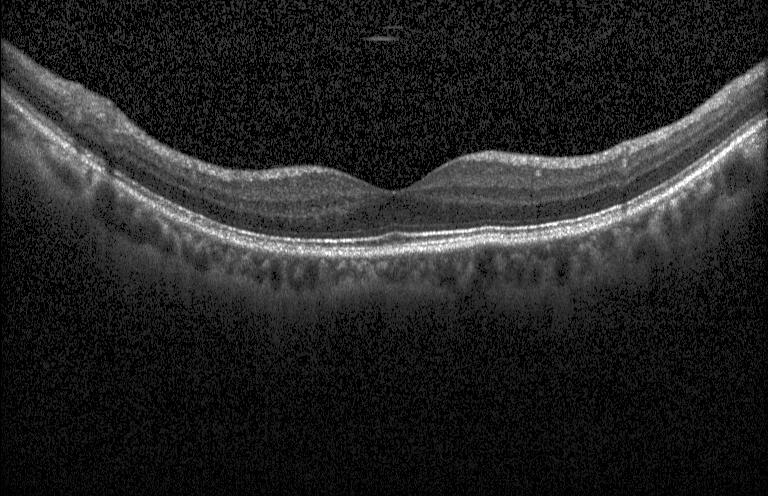 Acquired on a Heidelberg Spectralis · OCT B-scan
No evidence of choroidal neovascularization, diabetic macular edema, or drusen.